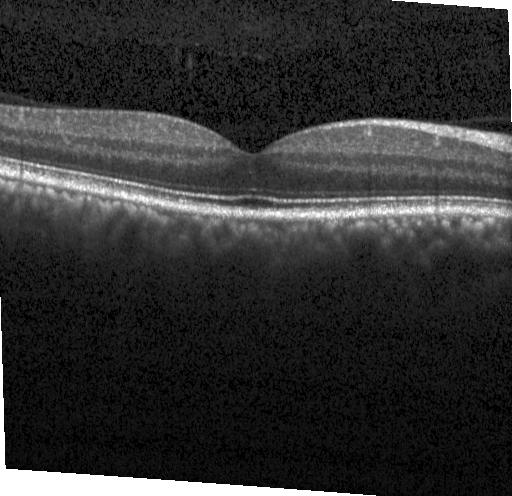 Macular OCT demonstrating no choroidal neovascularization, diabetic macular edema, or drusen.